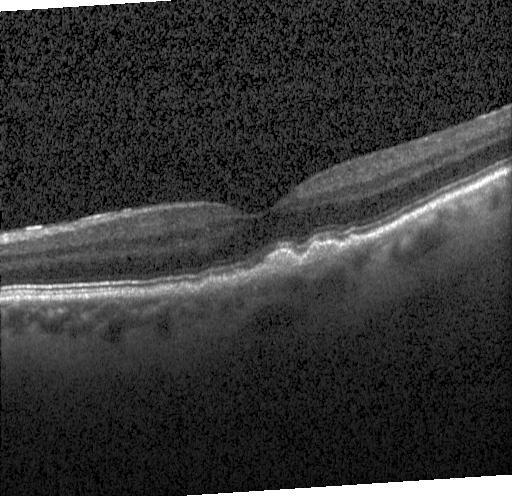

Retinal OCT B-scan · SD-OCT — The scan shows sub-RPE drusenoid deposits.